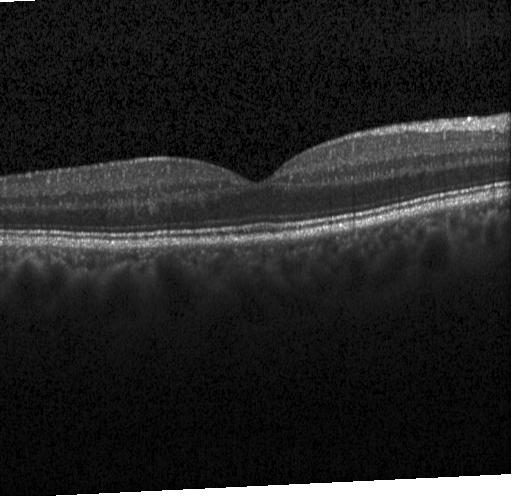

OCT line scan. Diagnosis: neither choroidal neovascularization, diabetic macular edema, nor drusen.